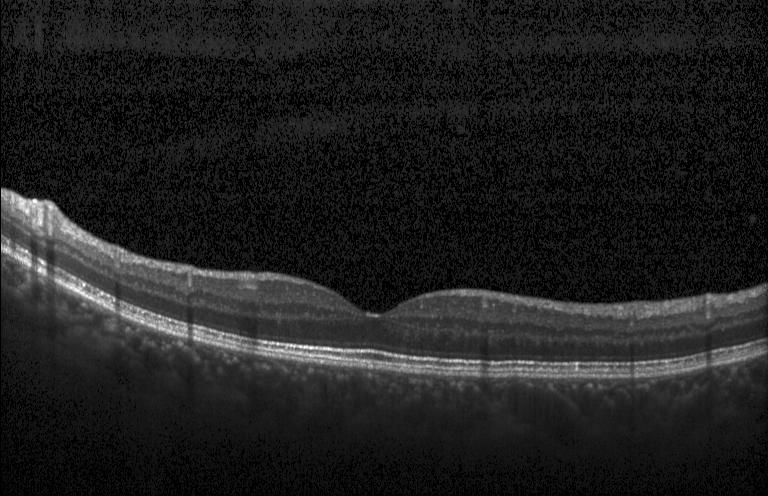
Acquired on a Heidelberg Spectralis · spectral-domain OCT · retinal OCT B-scan · through the macula.
Finding: no CNV, no DME, and no drusen.